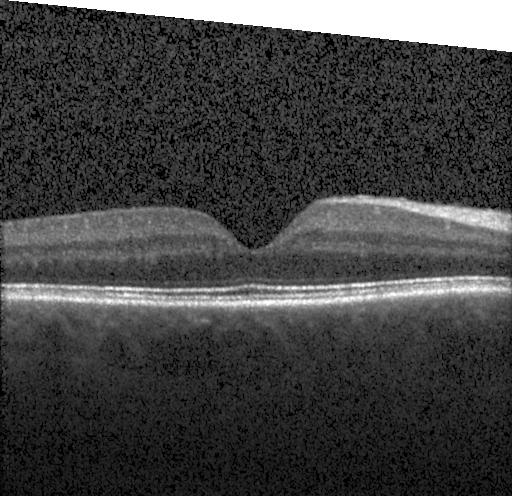

Impression: no choroidal neovascularization, diabetic macular edema, or drusen.